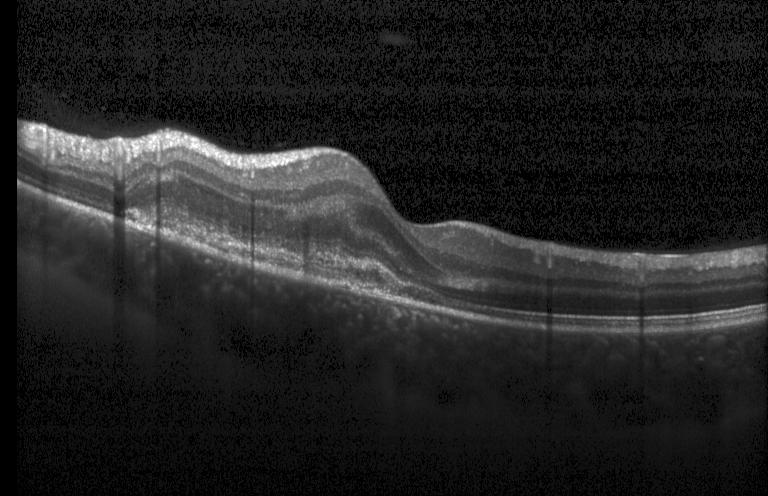

Optical coherence tomography scan.
Dx: a choroidal neovascular membrane.